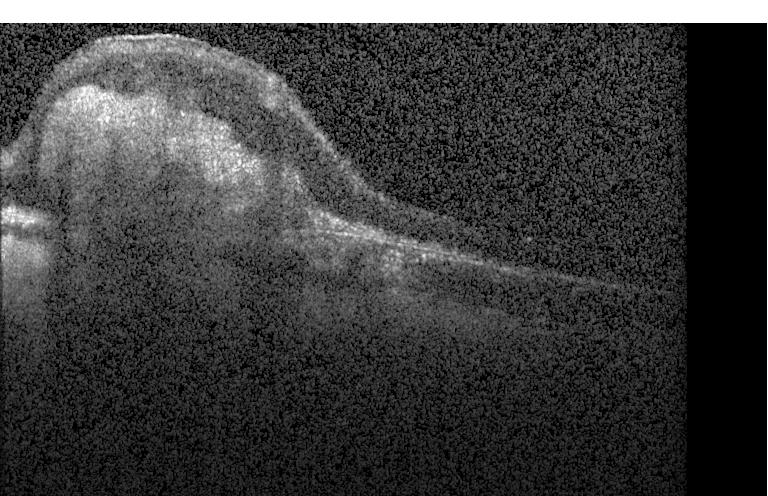
SD-OCT. Through the macula. Retinal OCT B-scan — The scan shows choroidal neovascularization.